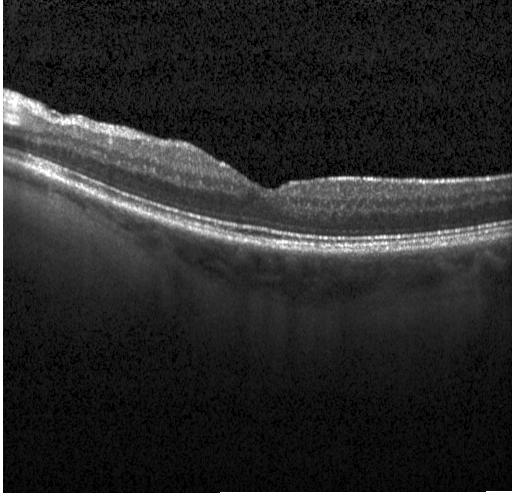
This B-scan demonstrates no choroidal neovascularization, diabetic macular edema, or drusen.